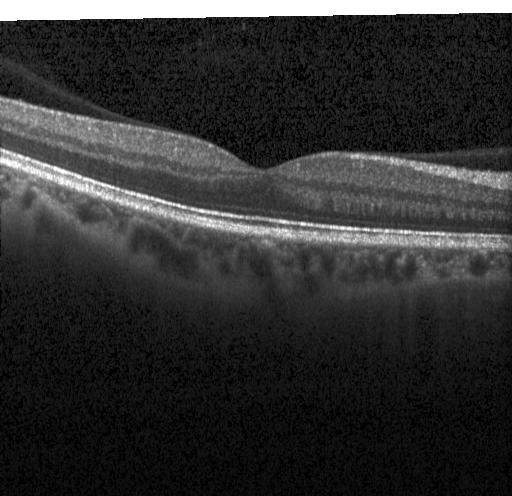

Heidelberg Spectralis; through the macula; optical coherence tomography scan; spectral-domain optical coherence tomography — Diagnosis: neither choroidal neovascularization, diabetic macular edema, nor drusen.